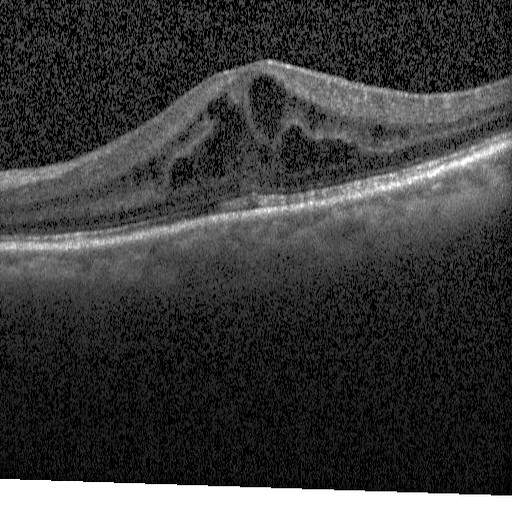
This B-scan demonstrates diabetic macular edema.